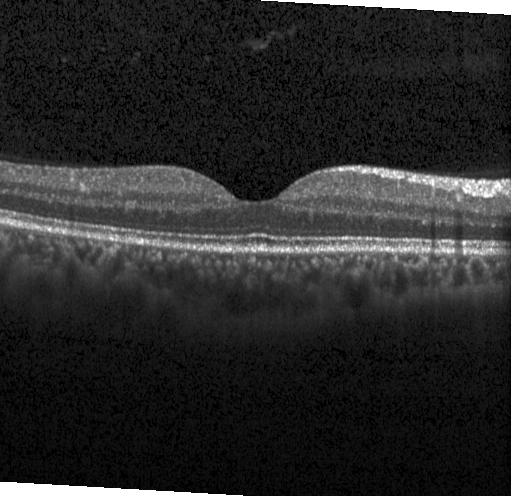 Retinal OCT B-scan
Assessment: neither choroidal neovascularization, diabetic macular edema, nor drusen.